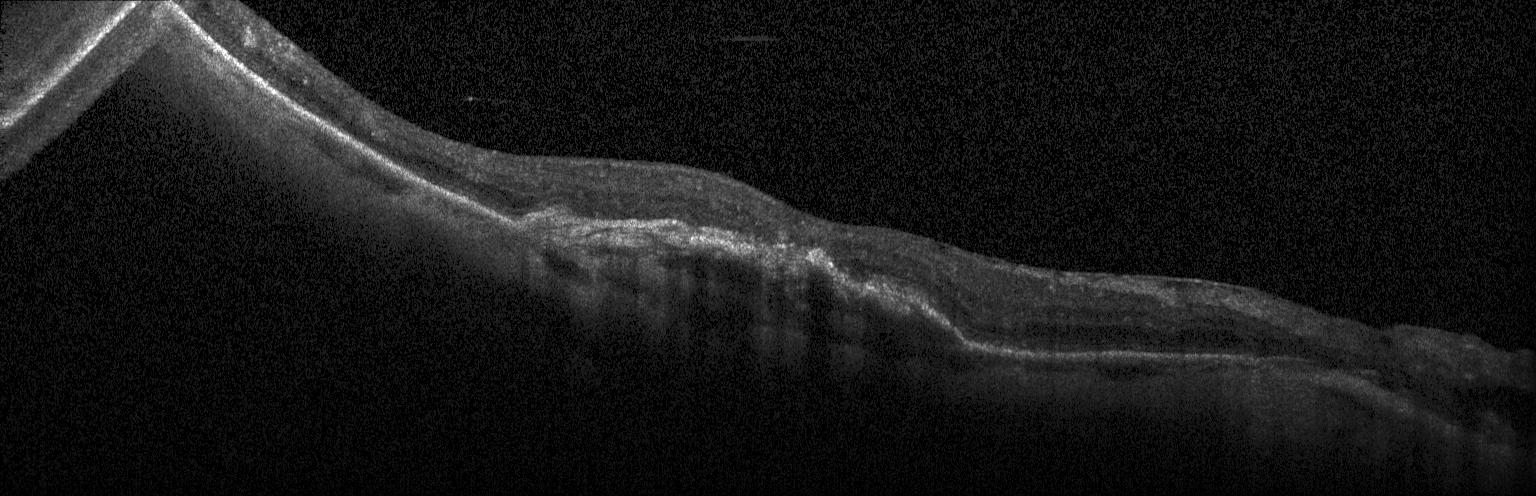
Diagnosis: CNV.